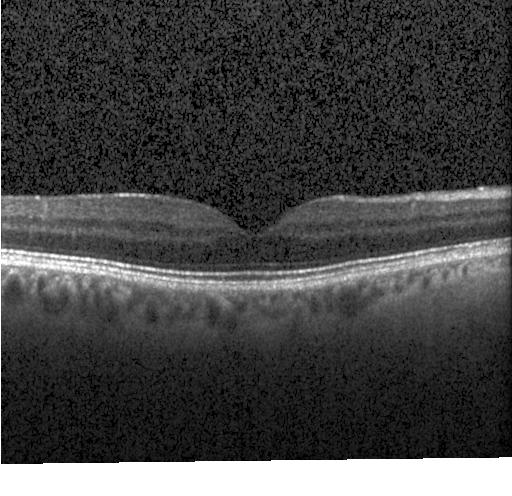

Optical coherence tomography scan; acquired on a Heidelberg Spectralis; spectral-domain OCT; macular scan
This B-scan demonstrates no CNV, DME, or drusen.